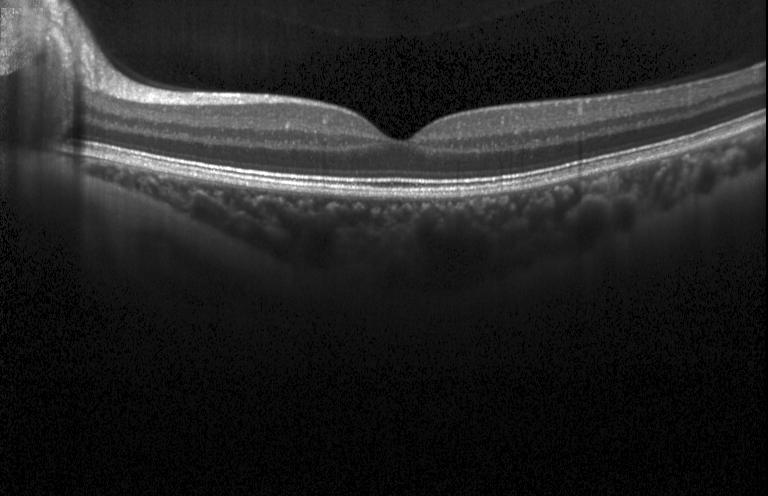

Retinal OCT cross-section · instrument: Heidelberg Spectralis · centered on the fovea. Macular OCT: neither choroidal neovascularization, diabetic macular edema, nor drusen.